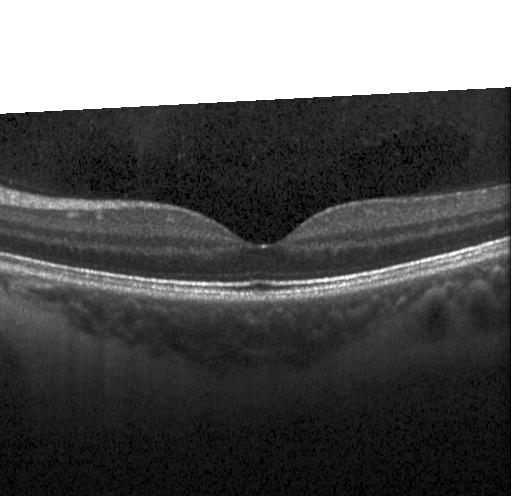 Optical coherence tomography scan, SD-OCT, acquired on a Heidelberg Spectralis — This B-scan demonstrates no evidence of CNV, DME, or drusen.